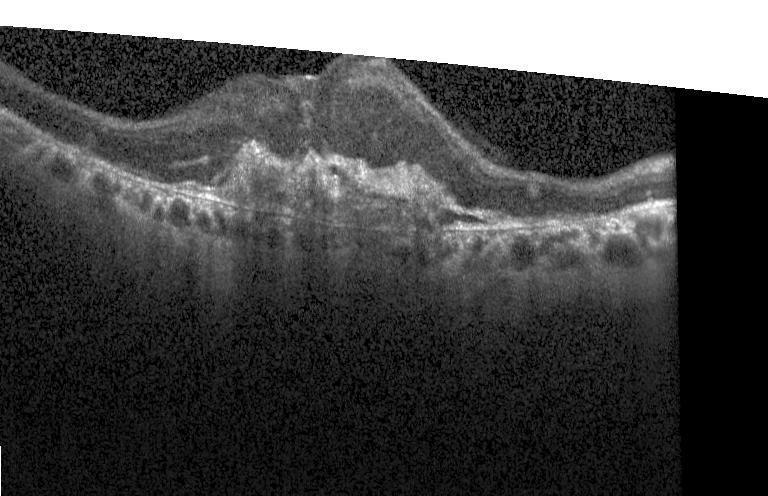
OCT line scan.
Finding: CNV.